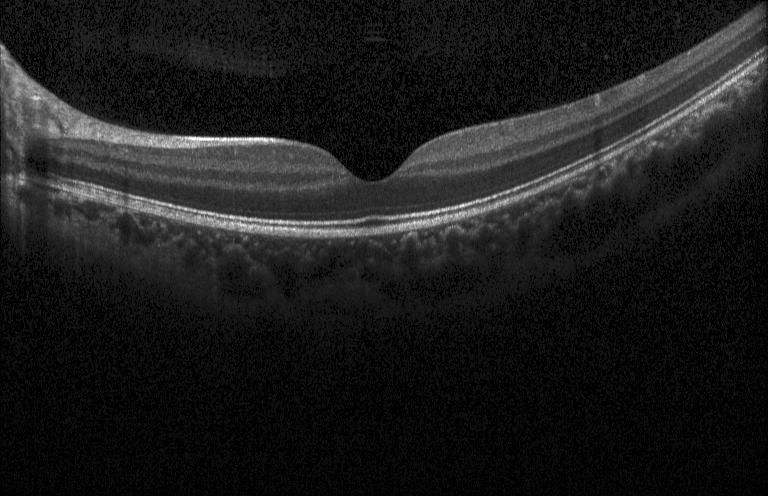
Heidelberg Spectralis OCT system, horizontal scan through the fovea, SD-OCT, optical coherence tomography scan.
Diagnosis: neither choroidal neovascularization, diabetic macular edema, nor drusen.